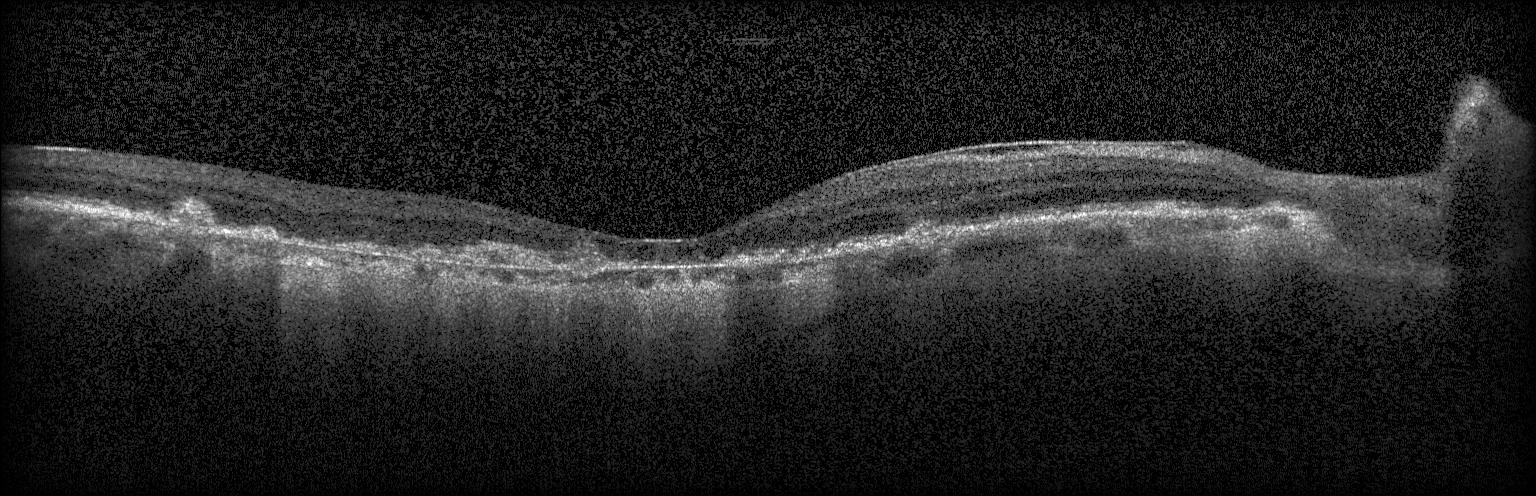
OCT B-scan
The scan shows choroidal neovascularization (CNV).